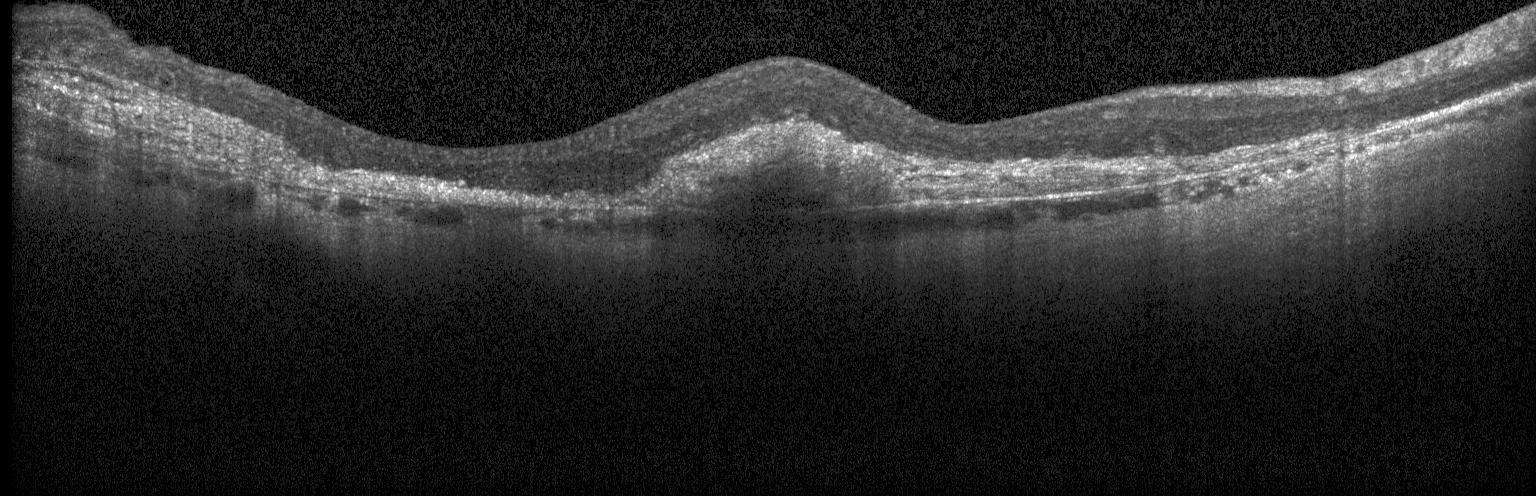 Spectral-domain OCT B-scan: a choroidal neovascular membrane.